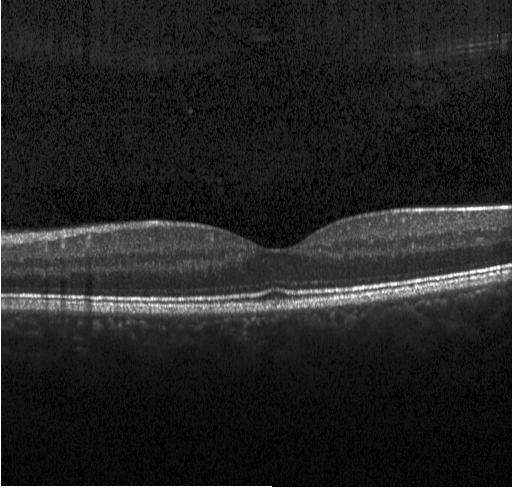
Spectral-domain OCT B-scan: no evidence of choroidal neovascularization, diabetic macular edema, or drusen.